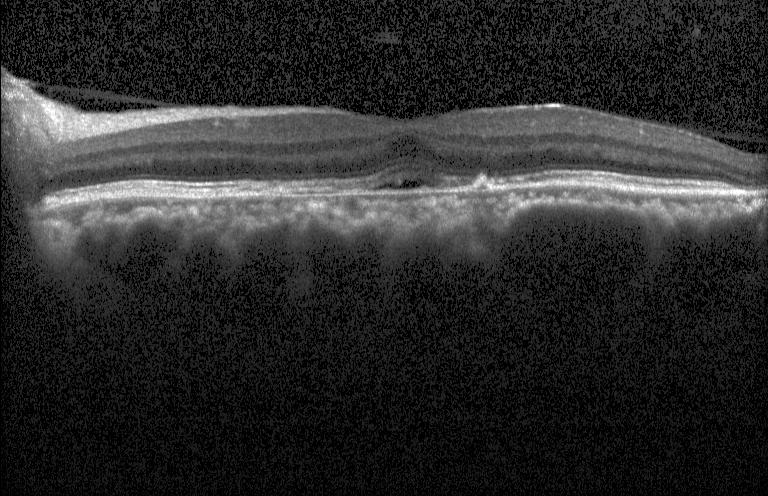 Impression: a choroidal neovascular membrane.